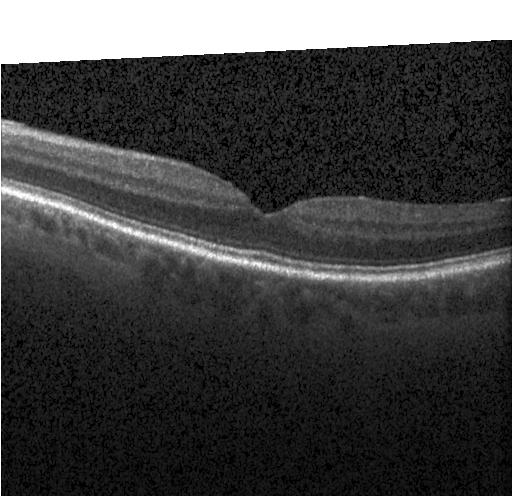
Instrument: Heidelberg Spectralis; SD-OCT; optical coherence tomography B-scan
Finding: no evidence of CNV, DME, or drusen.